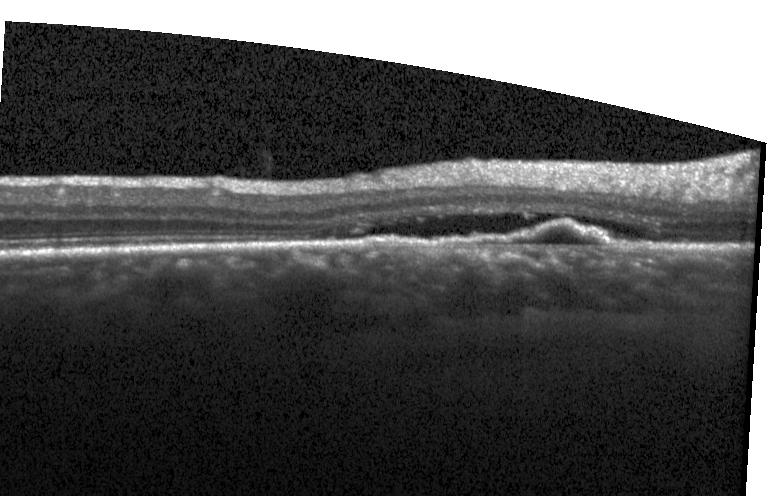 Through the macula; retinal OCT cross-section — Finding: CNV.